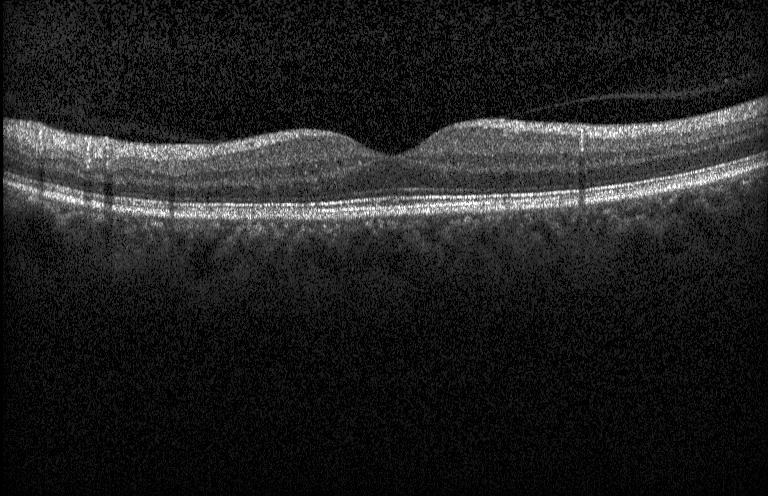 The scan shows neither CNV, DME, nor drusen.